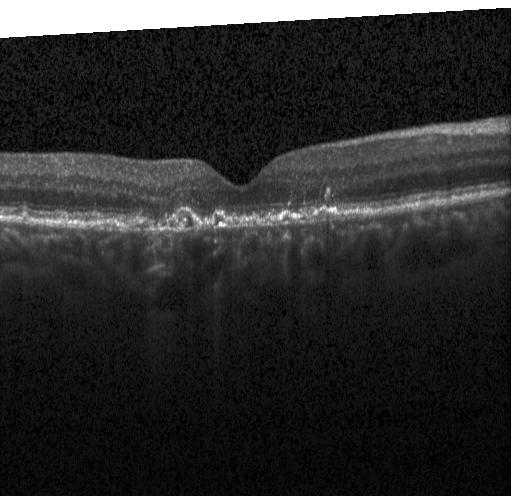

Dx: choroidal neovascularization (CNV).